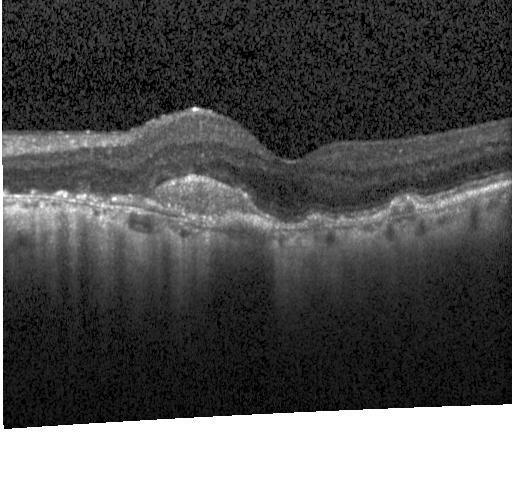
OCT B-scan. Spectral-domain OCT. Instrument: Heidelberg Spectralis. This B-scan demonstrates a choroidal neovascular membrane.